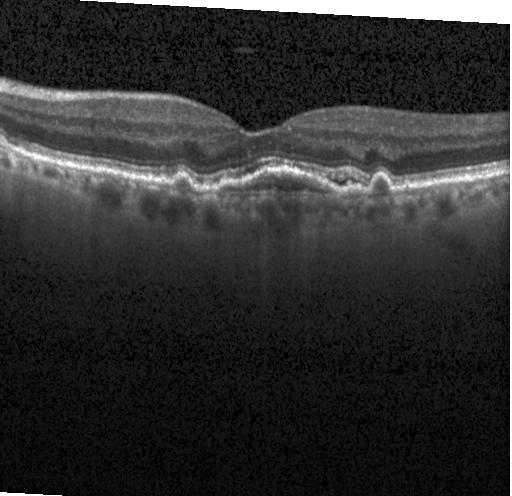

OCT B-scan showing CNV.